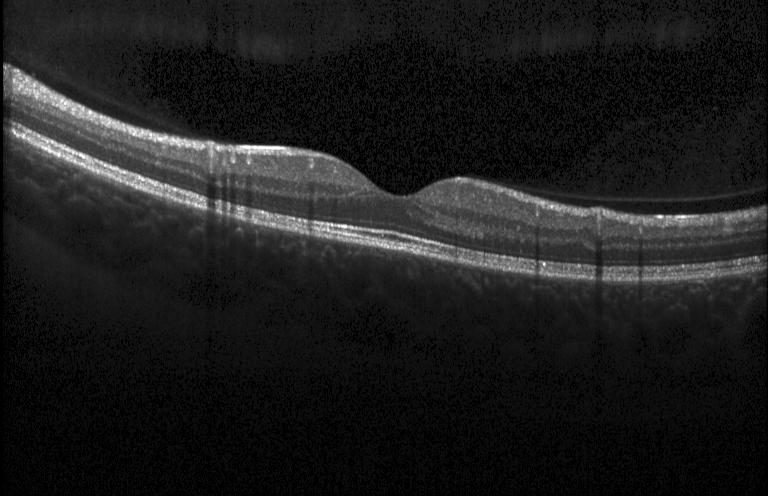 Retinal OCT cross-section · spectral-domain optical coherence tomography · acquired on a Heidelberg Spectralis · through the macula. Impression: neither CNV, DME, nor drusen.